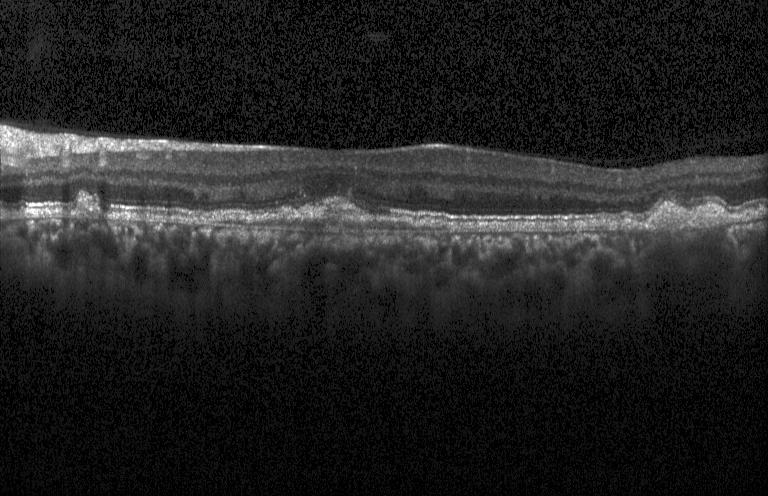

OCT scan showing choroidal neovascularization (CNV).